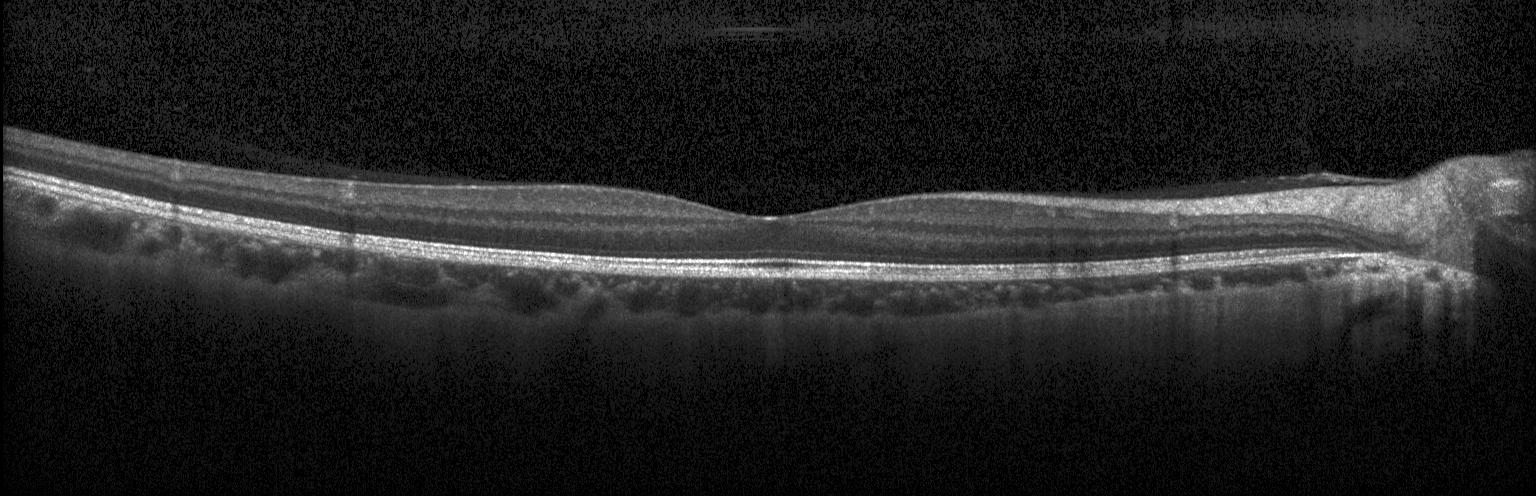

OCT B-scan
This B-scan demonstrates no evidence of CNV, DME, or drusen.